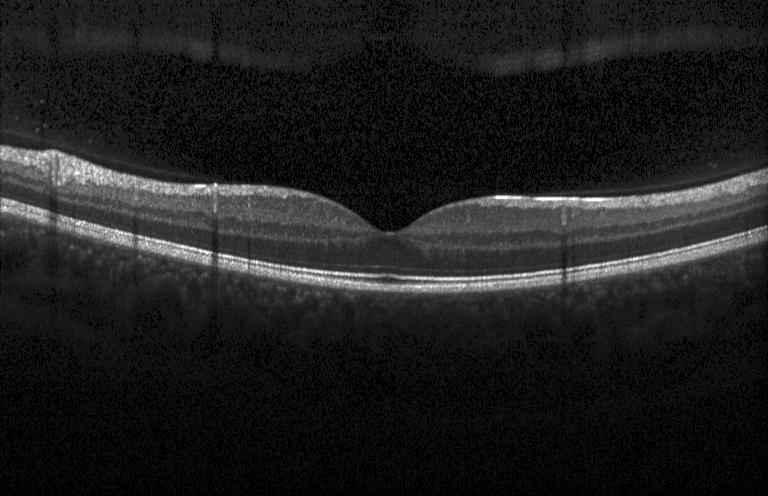 OCT B-scan — No choroidal neovascularization, diabetic macular edema, or drusen.